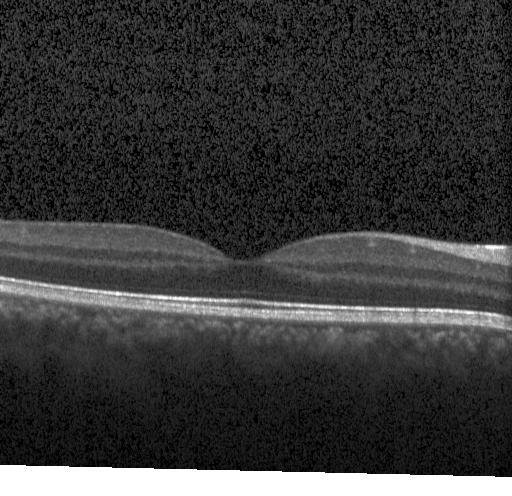
Dx: no choroidal neovascularization, diabetic macular edema, or drusen.